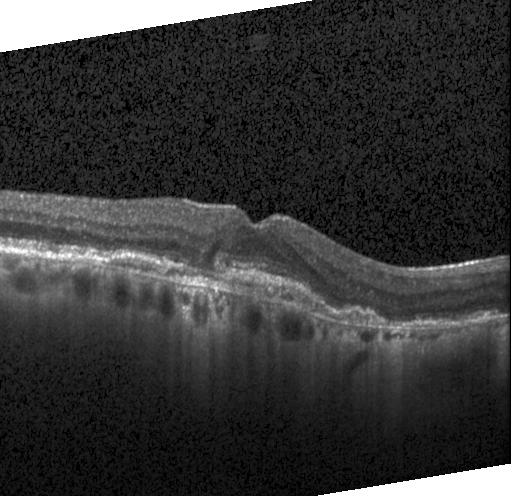

Retinal OCT cross-section showing choroidal neovascularization (CNV).